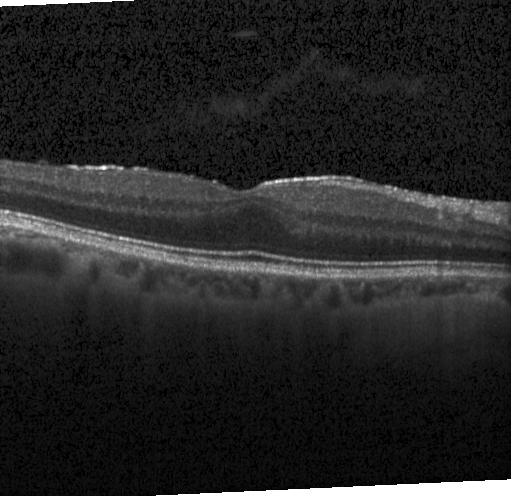
Horizontal scan through the fovea, retinal OCT cross-section.
Assessment: no evidence of choroidal neovascularization, diabetic macular edema, or drusen.